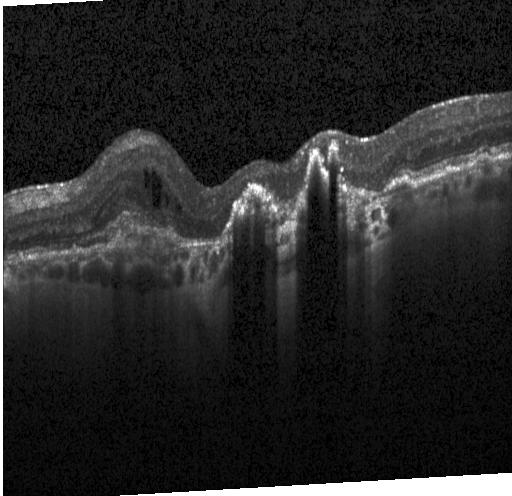
Optical coherence tomography scan. Finding: choroidal neovascularization (CNV).